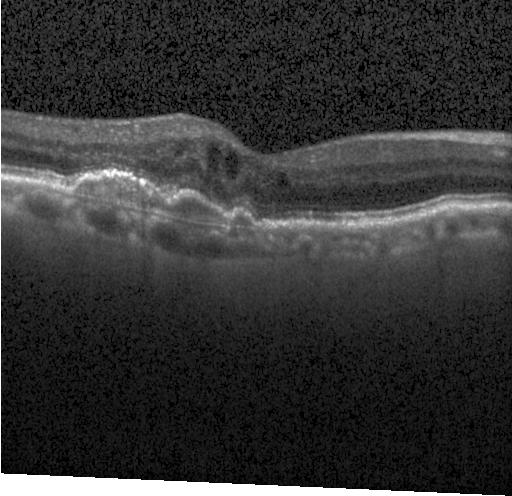

Through the macula; Heidelberg Spectralis; spectral-domain OCT; optical coherence tomography B-scan.
OCT finding: choroidal neovascularization.